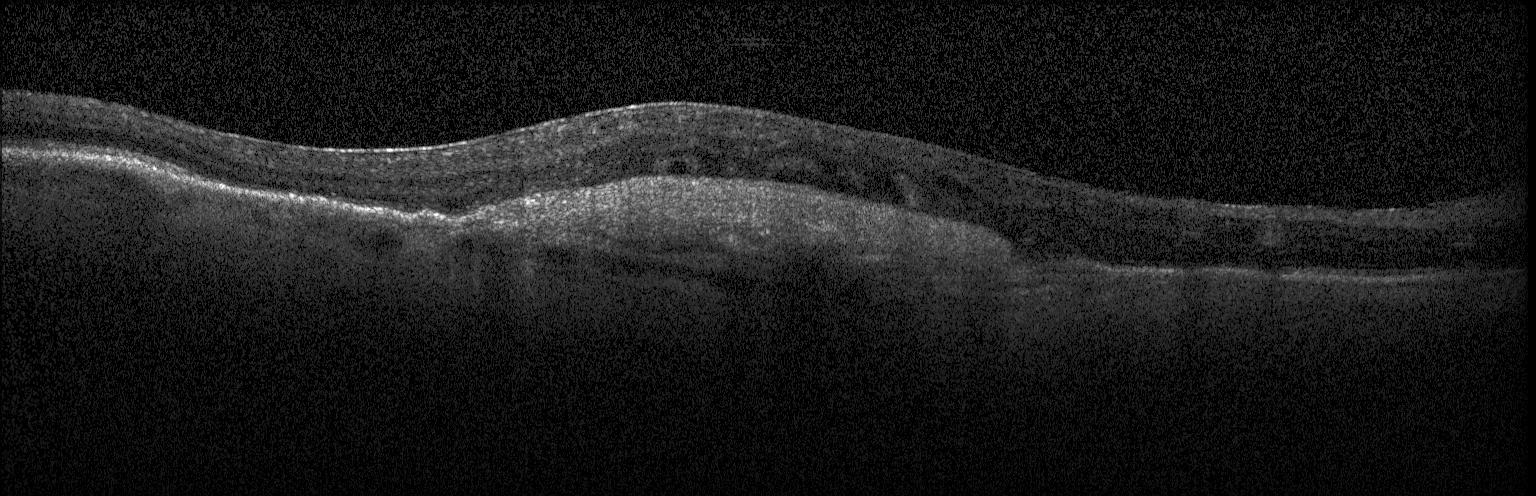
Dx: a choroidal neovascular membrane.